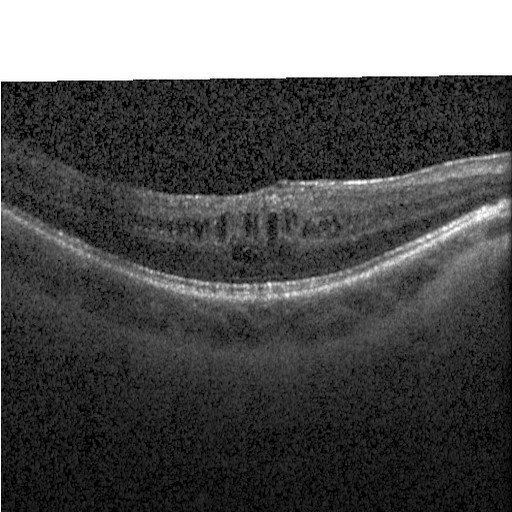
OCT finding: diabetic macular edema.